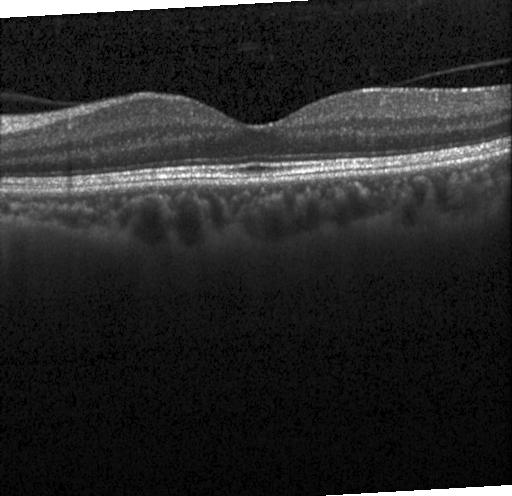
Spectral-domain optical coherence tomography; retinal OCT B-scan — This B-scan demonstrates no choroidal neovascularization, no diabetic macular edema, and no drusen.